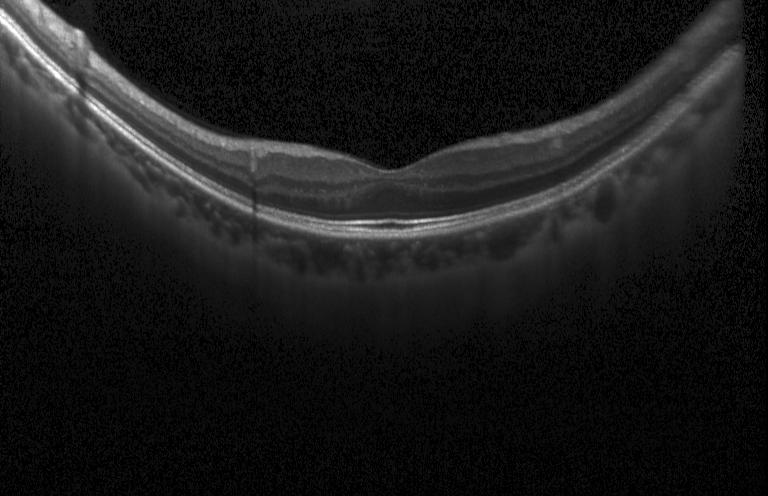 OCT finding: no choroidal neovascularization, diabetic macular edema, or drusen.